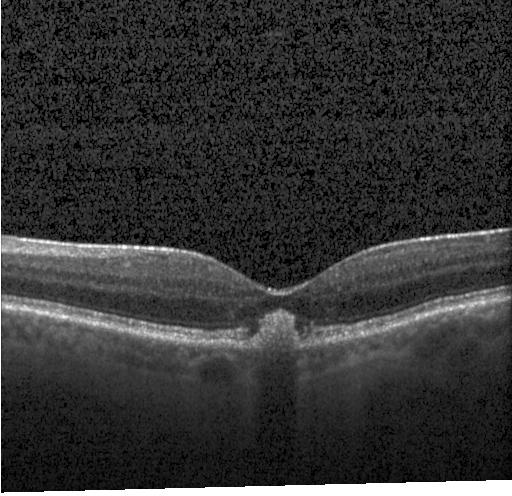

Fovea-centered. Spectral-domain optical coherence tomography. Optical coherence tomography scan. Heidelberg Spectralis — A choroidal neovascular membrane.